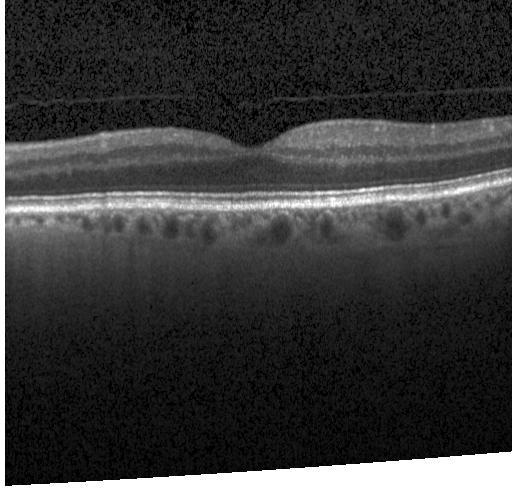
Spectral-domain optical coherence tomography · acquired on a Heidelberg Spectralis · retinal OCT B-scan · fovea-centered
Dx: no evidence of choroidal neovascularization, diabetic macular edema, or drusen.